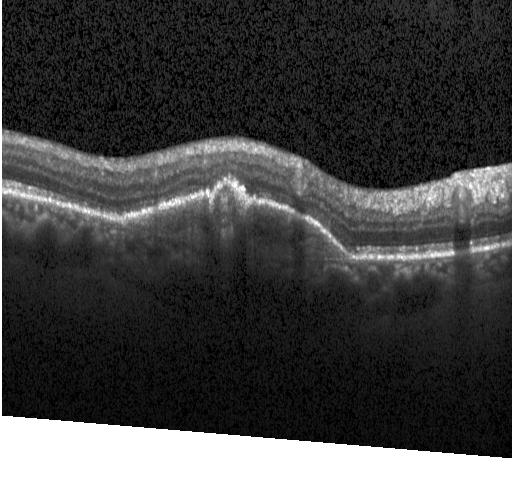 Spectral-domain OCT. OCT B-scan
OCT finding: a choroidal neovascular membrane.